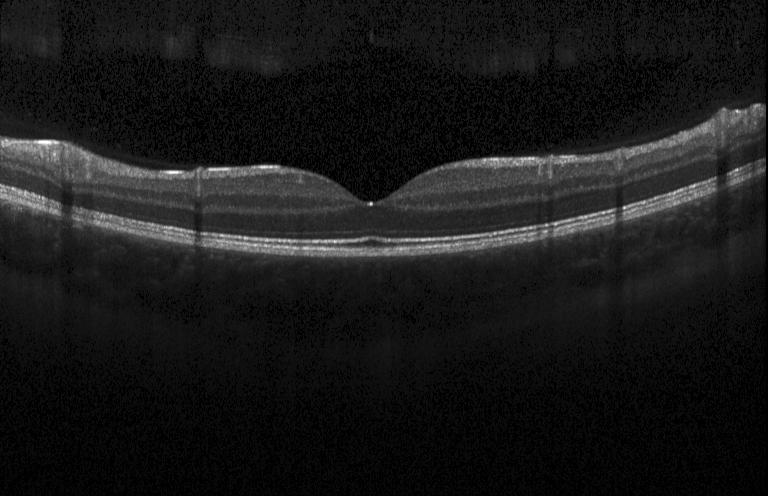 Retinal OCT B-scan.
Diagnosis: no choroidal neovascularization, no diabetic macular edema, and no drusen.